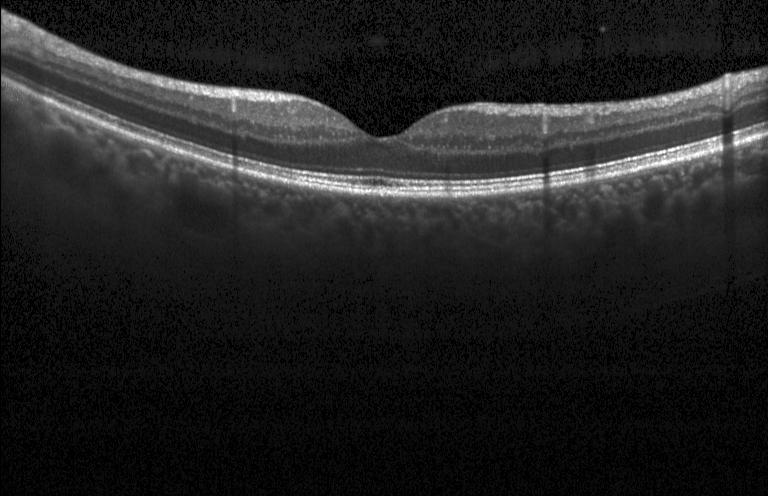 Acquired on a Heidelberg Spectralis, OCT B-scan
This B-scan demonstrates no choroidal neovascularization, diabetic macular edema, or drusen.